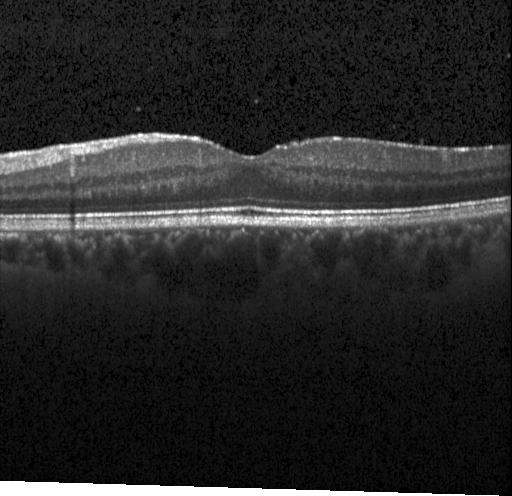 Retinal OCT B-scan; SD-OCT; through the macula; acquired on a Heidelberg Spectralis.
Assessment: no CNV, DME, or drusen.